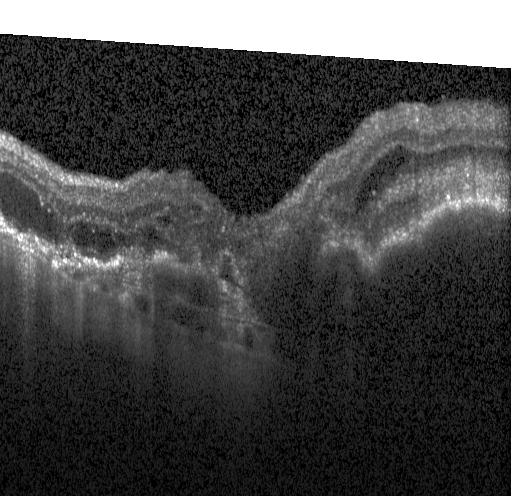
Assessment: a choroidal neovascular membrane.